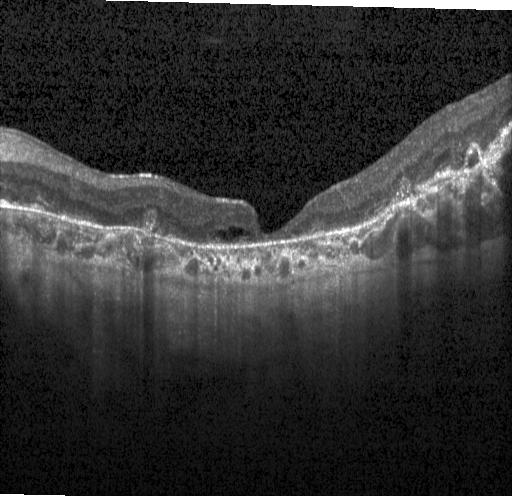

Horizontal scan through the fovea. Retinal OCT cross-section — This B-scan demonstrates choroidal neovascularization.